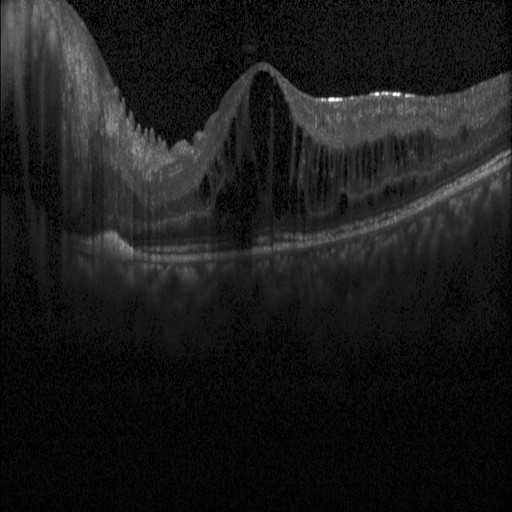

Impression: DME.